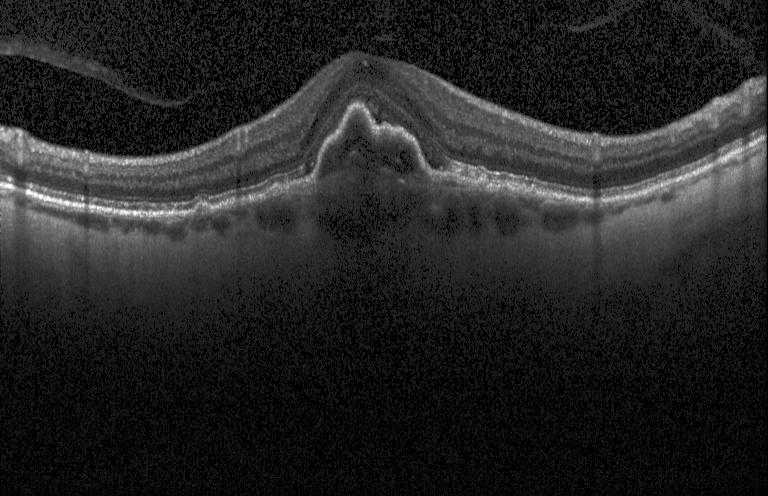
Spectral-domain OCT B-scan: choroidal neovascularization.